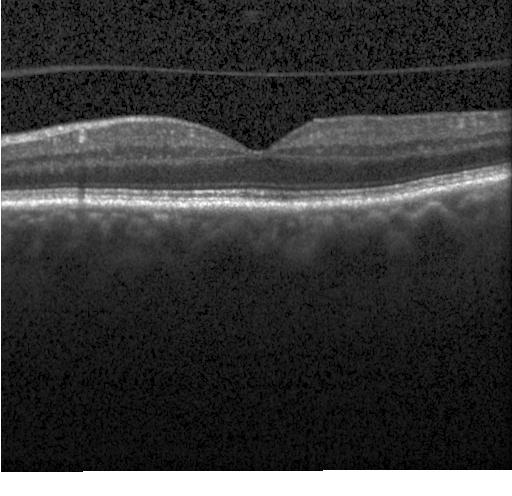
Heidelberg Spectralis OCT system. Retinal OCT cross-section. SD-OCT.
This B-scan demonstrates no evidence of choroidal neovascularization, diabetic macular edema, or drusen.